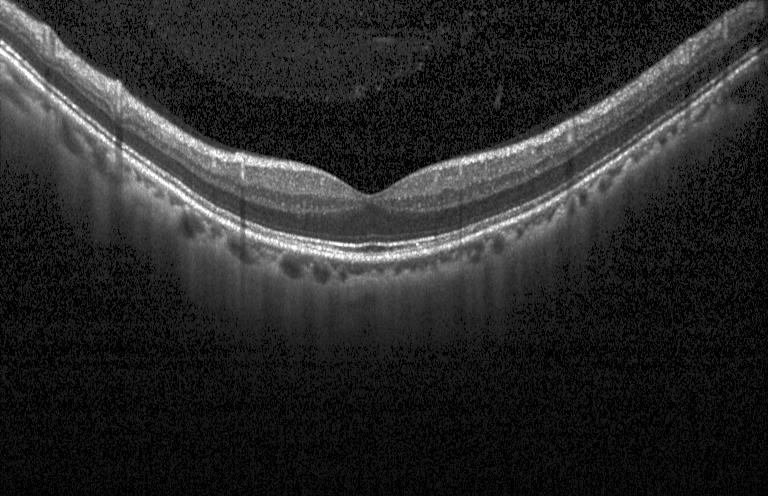

Retinal OCT B-scan
Diagnosis: no evidence of choroidal neovascularization, diabetic macular edema, or drusen.